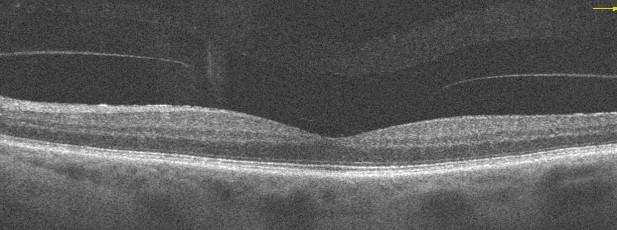
OCT B-scan showing absence of AMD, DME, ERM, RAO, RVO, and vitreomacular interface disease.